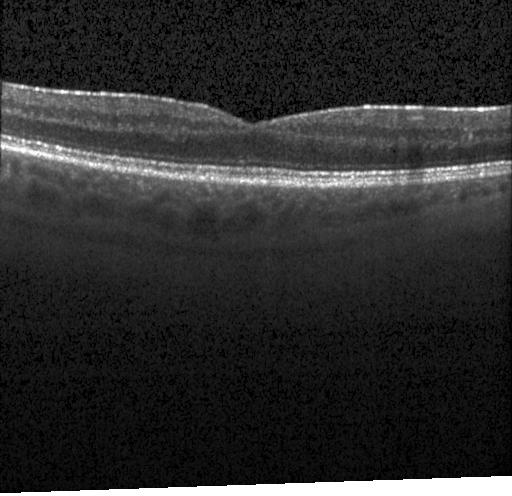

Assessment: no choroidal neovascularization, diabetic macular edema, or drusen.